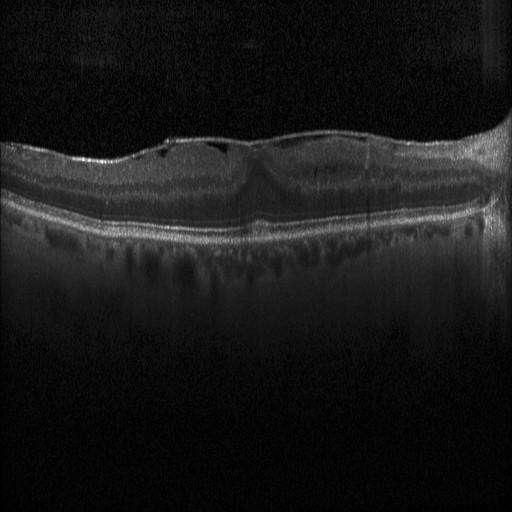 Optical coherence tomography B-scan. Finding: diabetic macular edema (DME).